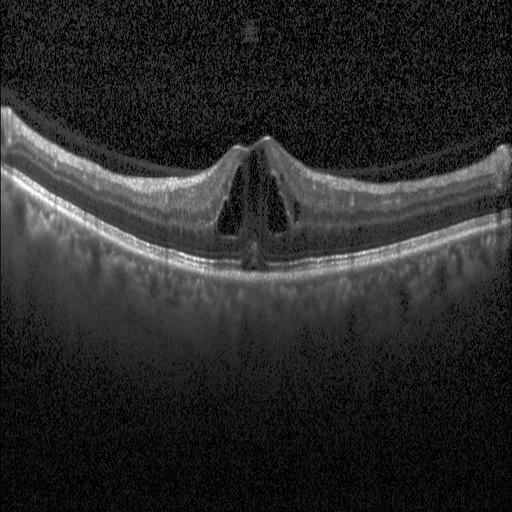

Optical coherence tomography B-scan. The scan shows diabetic macular edema (DME).